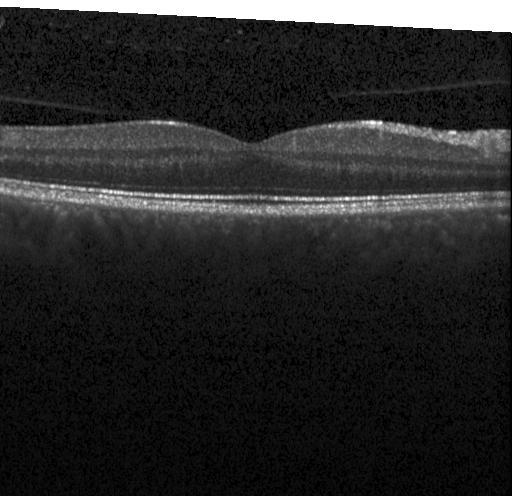 SD-OCT, OCT line scan, through the macula, acquired on a Heidelberg Spectralis.
The scan shows no choroidal neovascularization, no diabetic macular edema, and no drusen.